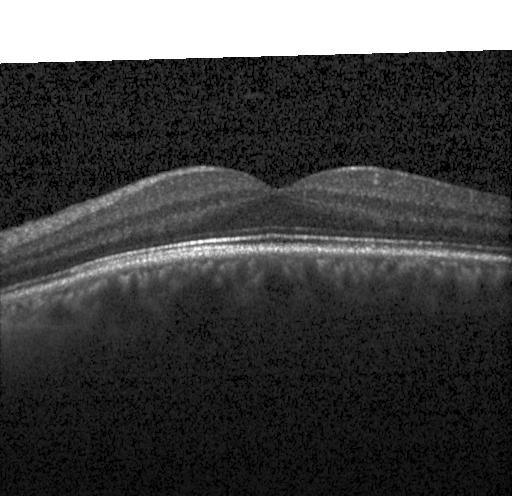

Optical coherence tomography scan — Dx: no evidence of CNV, DME, or drusen.